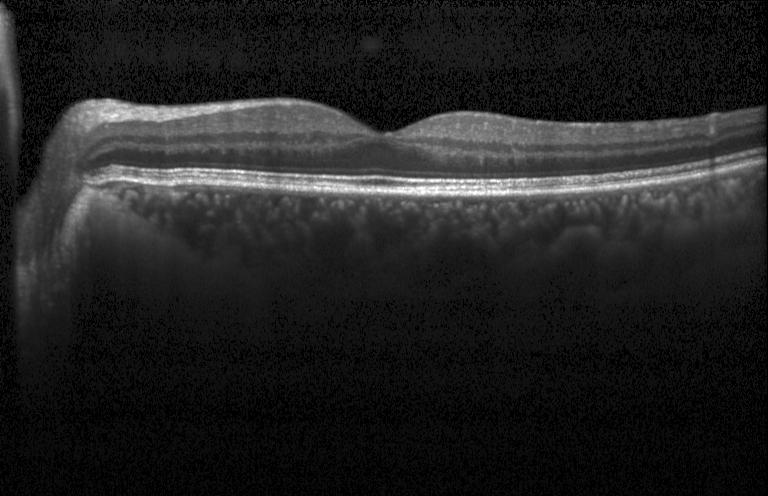
Finding: no choroidal neovascularization, no diabetic macular edema, and no drusen.